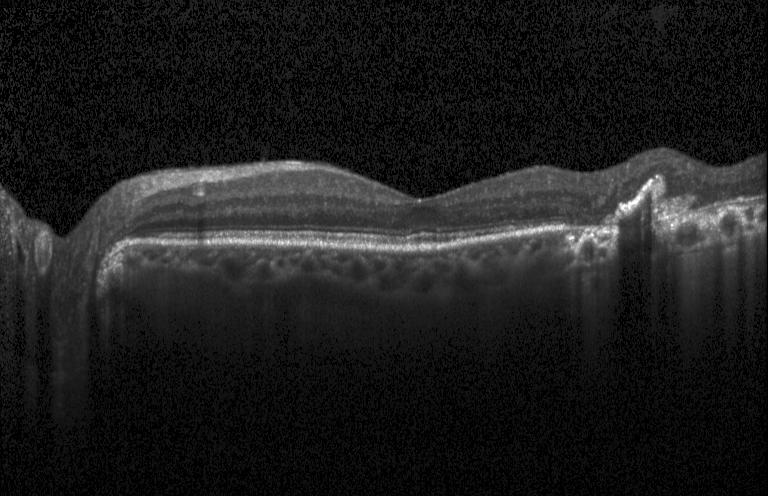 OCT B-scan. Diagnosis: a choroidal neovascular membrane.